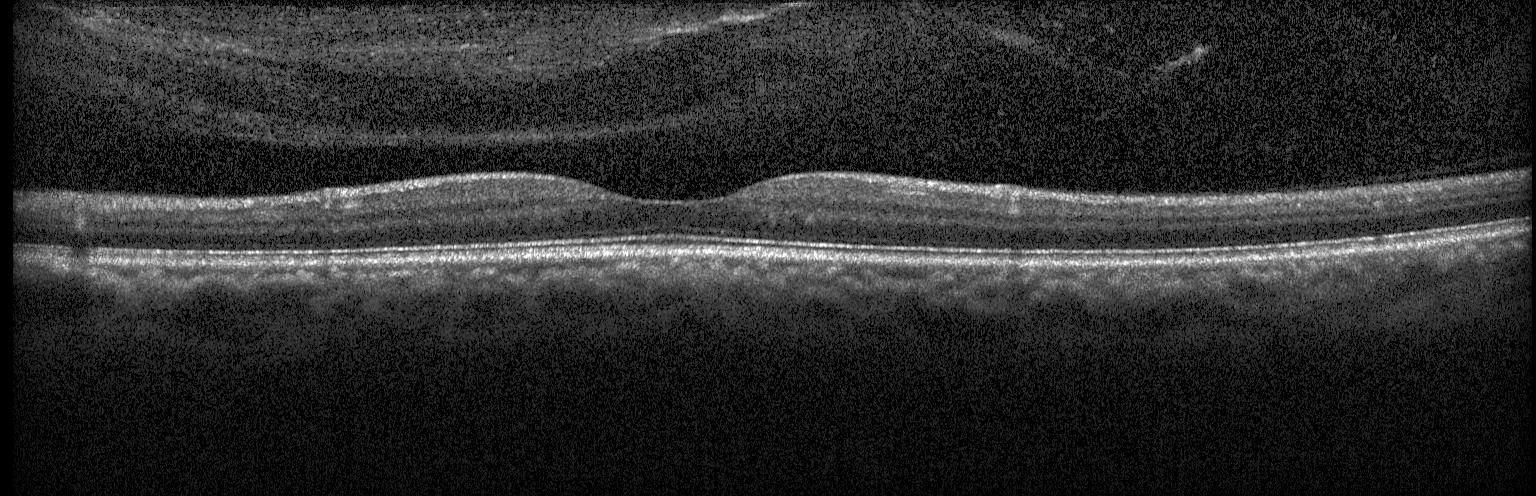
Diagnosis: no CNV, no DME, and no drusen.